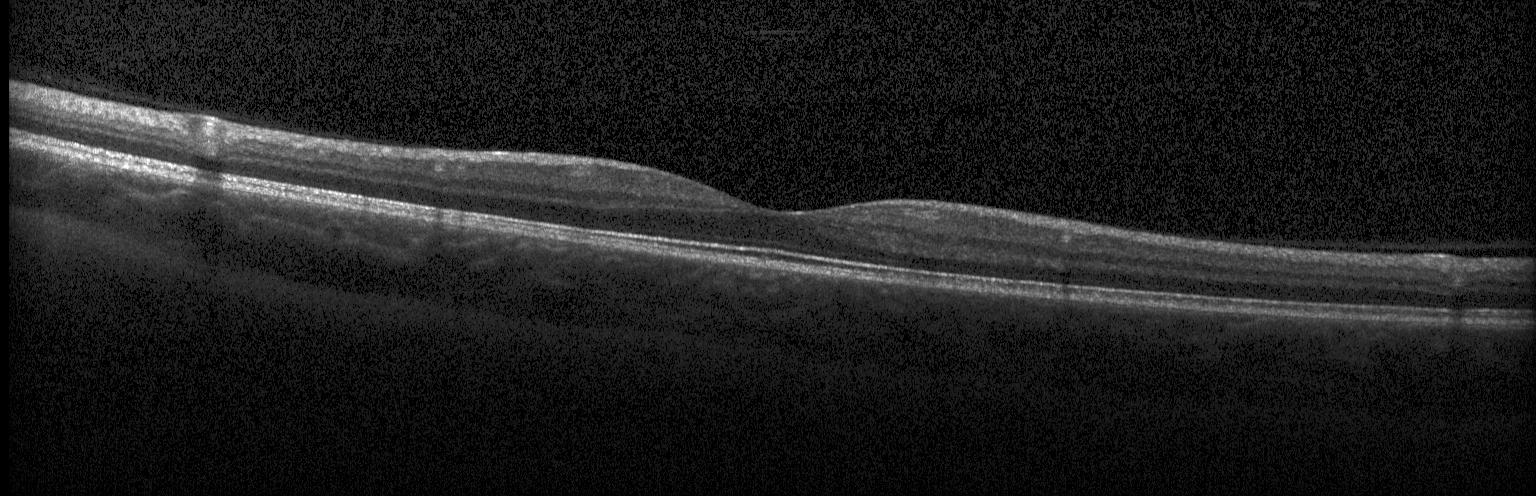

Finding: no CNV, no DME, and no drusen.